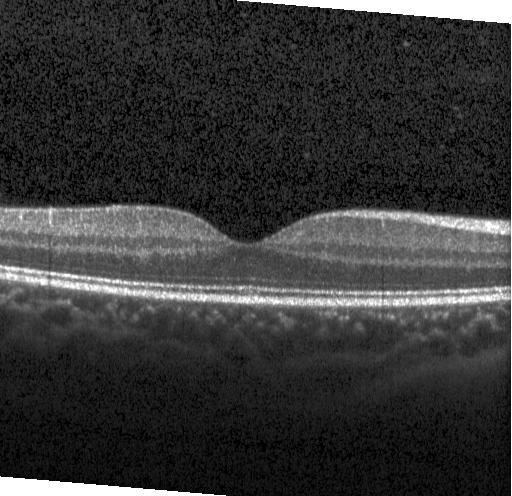

Through the macula, OCT B-scan
No choroidal neovascularization, no diabetic macular edema, and no drusen.